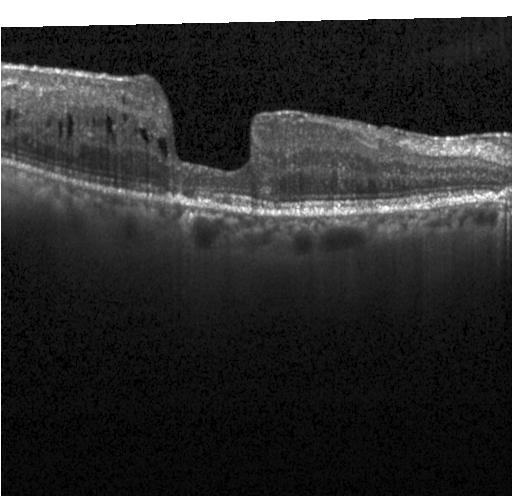
OCT B-scan — Finding: diabetic macular edema (DME).